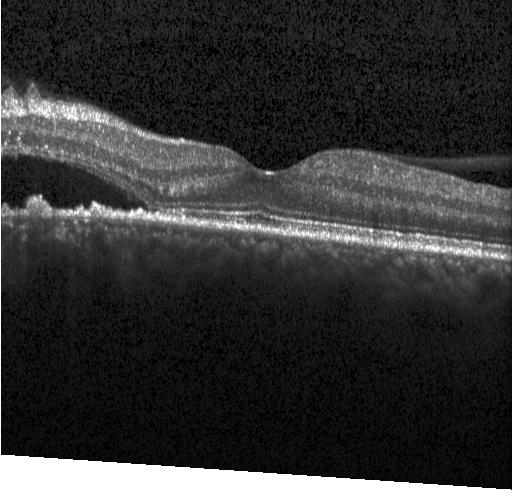

Optical coherence tomography scan.
OCT finding: a choroidal neovascular membrane.